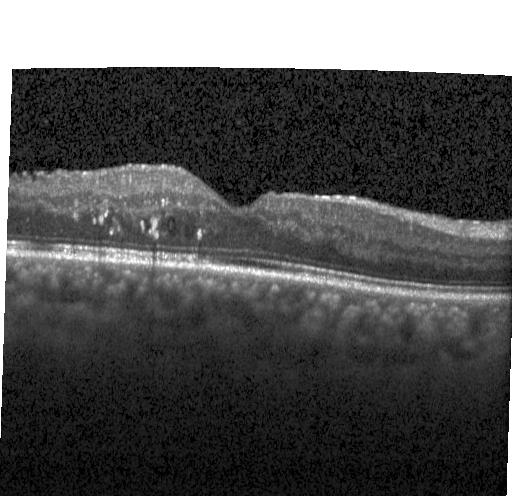

Retinal OCT cross-section
Impression: diabetic macular edema.